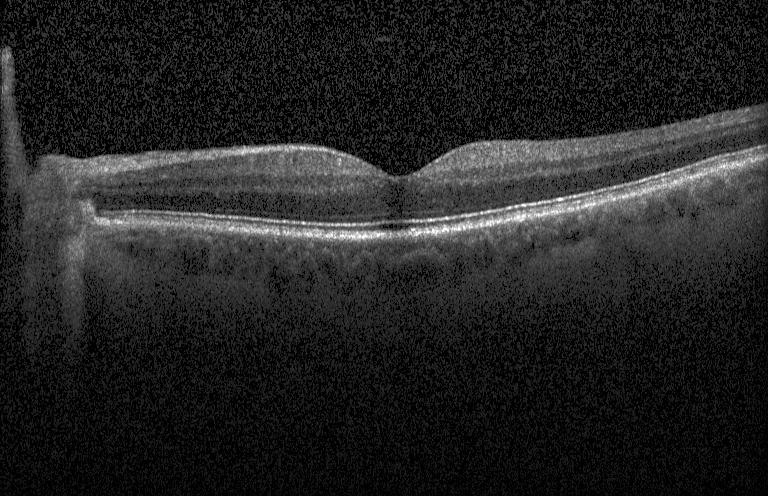
OCT line scan · acquired on a Heidelberg Spectralis · spectral-domain OCT. OCT finding: neither choroidal neovascularization, diabetic macular edema, nor drusen.